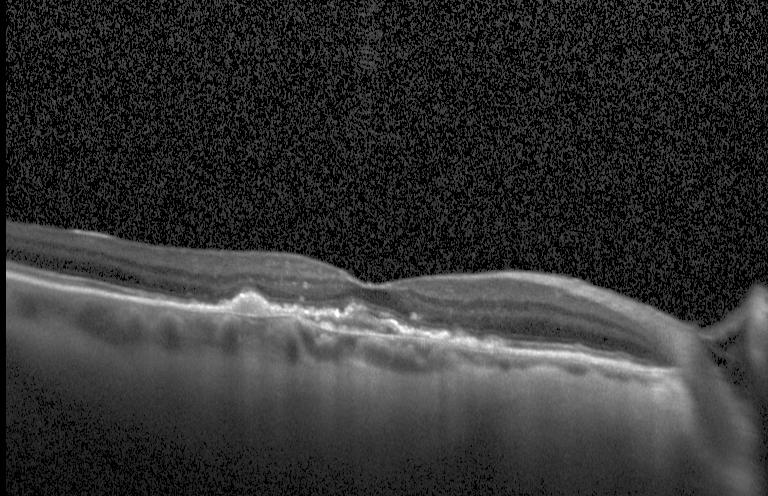
Finding: a choroidal neovascular membrane.